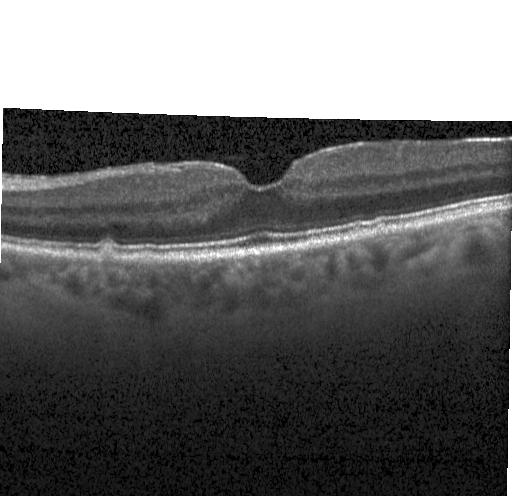

Horizontal scan through the fovea. SD-OCT. Optical coherence tomography B-scan. Diagnosis: multiple drusen.